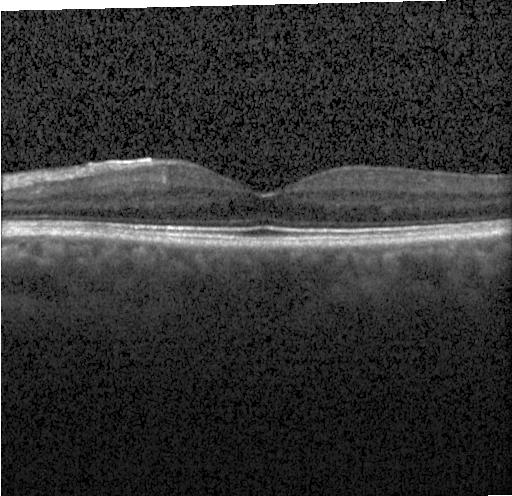

Spectral-domain OCT; through the macula; OCT line scan; Heidelberg Spectralis. Finding: neither choroidal neovascularization, diabetic macular edema, nor drusen.